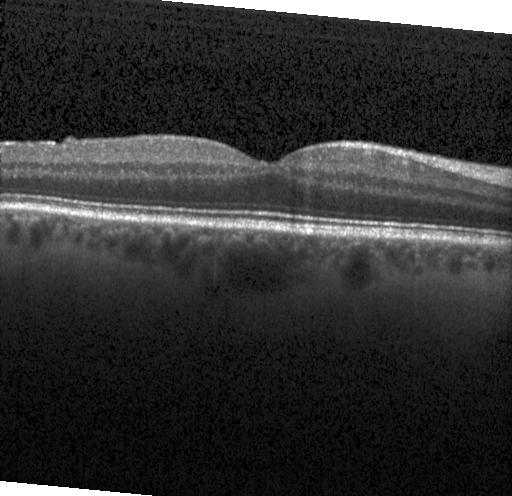
Macular OCT demonstrating no choroidal neovascularization, no diabetic macular edema, and no drusen.